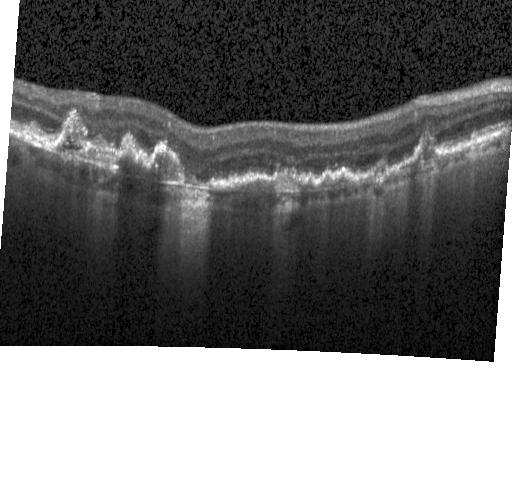

OCT line scan · spectral-domain optical coherence tomography — Finding: a choroidal neovascular membrane.